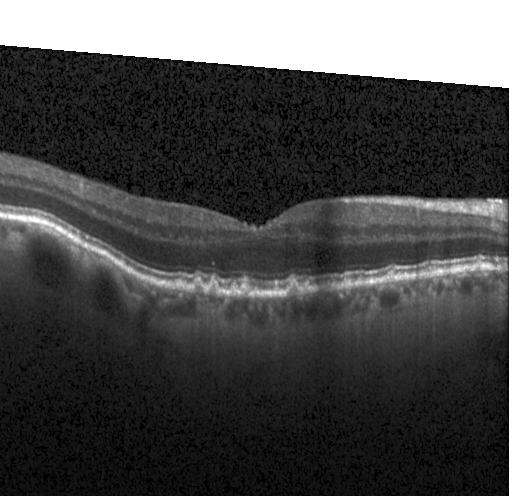 Retinal OCT B-scan; Heidelberg Spectralis; macular scan; SD-OCT — This B-scan demonstrates multiple drusen.